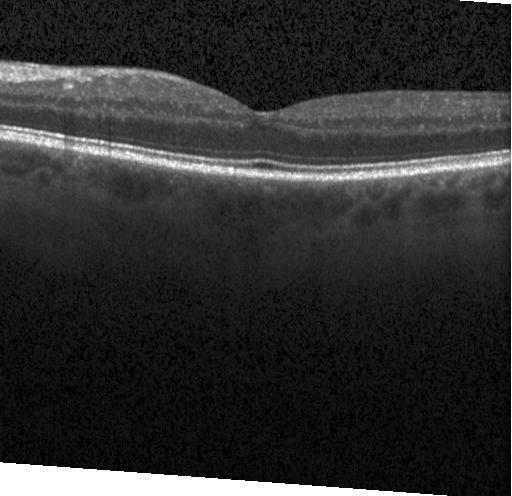

Fovea-centered · Heidelberg Spectralis OCT system · retinal OCT B-scan · spectral-domain OCT — Diagnosis: no choroidal neovascularization, no diabetic macular edema, and no drusen.